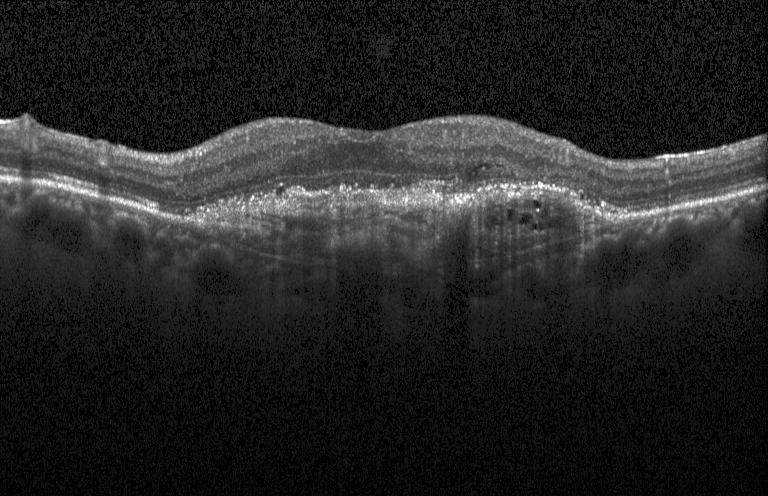 Finding: choroidal neovascularization (CNV).